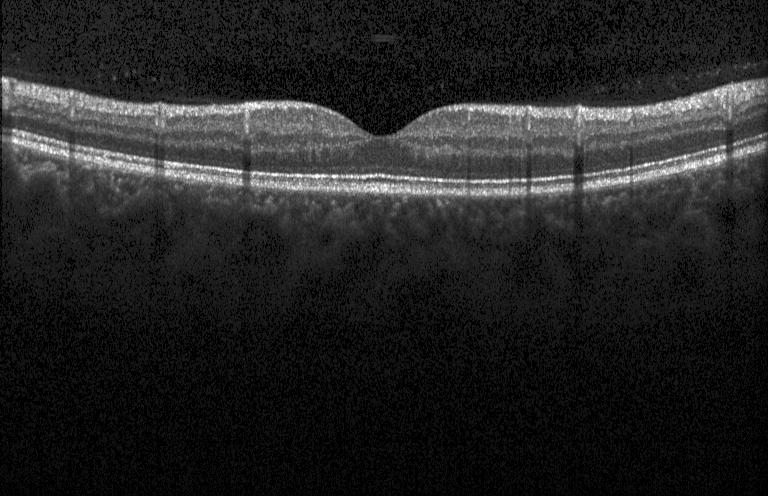 OCT line scan — Finding: no evidence of choroidal neovascularization, diabetic macular edema, or drusen.